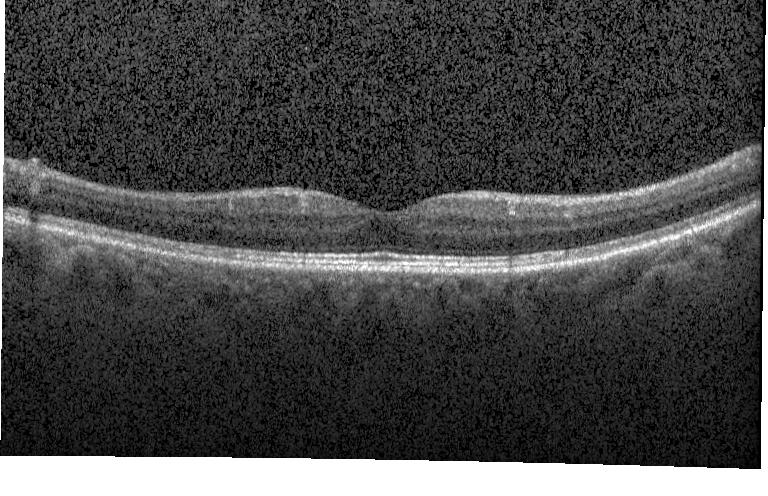

OCT line scan. Spectral-domain OCT — Assessment: neither choroidal neovascularization, diabetic macular edema, nor drusen.